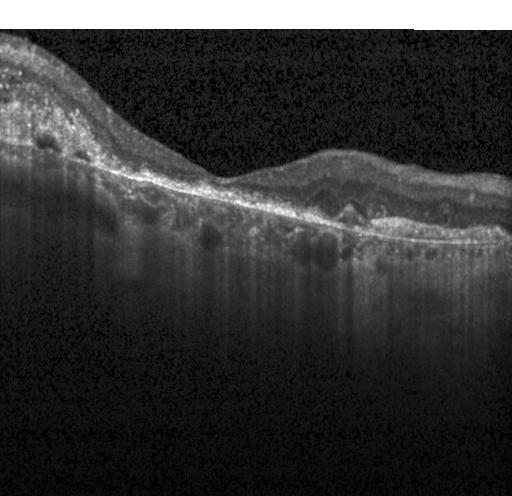

Diagnosis: choroidal neovascularization.